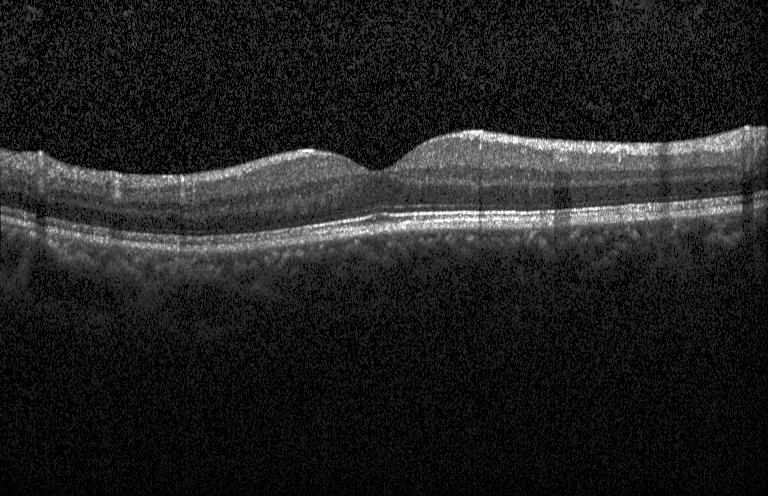

Instrument: Heidelberg Spectralis · retinal OCT cross-section · through the macula. This B-scan demonstrates neither CNV, DME, nor drusen.